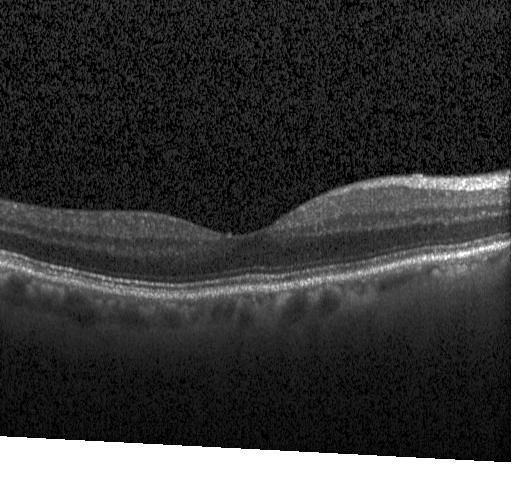
Optical coherence tomography B-scan.
Macular OCT: no evidence of CNV, DME, or drusen.